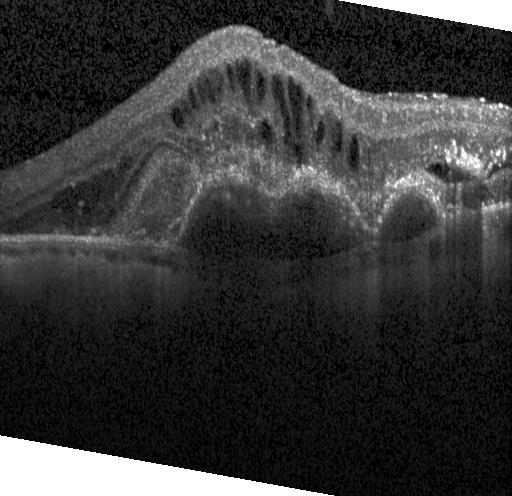 Optical coherence tomography scan. Dx: CNV.